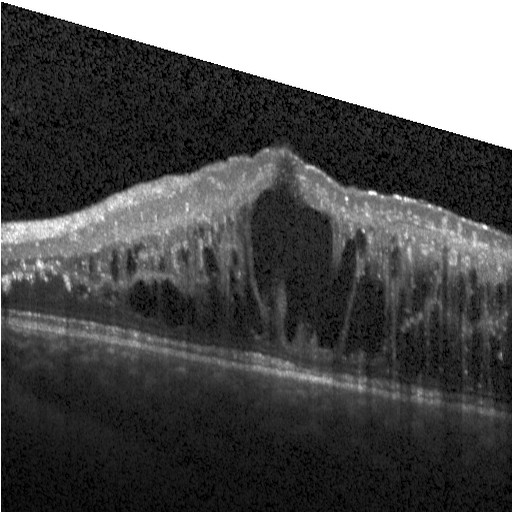
Impression: diabetic macular edema.